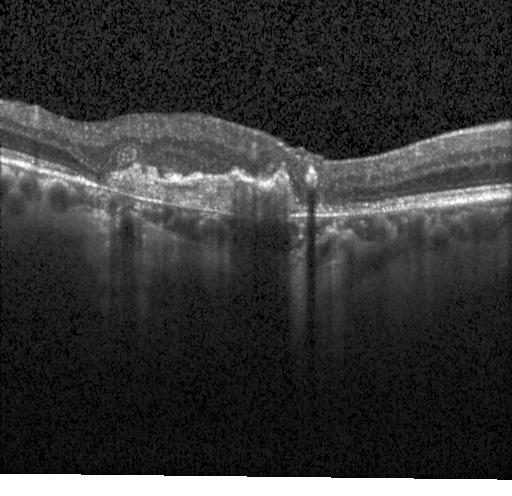
Horizontal scan through the fovea; Heidelberg Spectralis; OCT line scan. Finding: CNV.